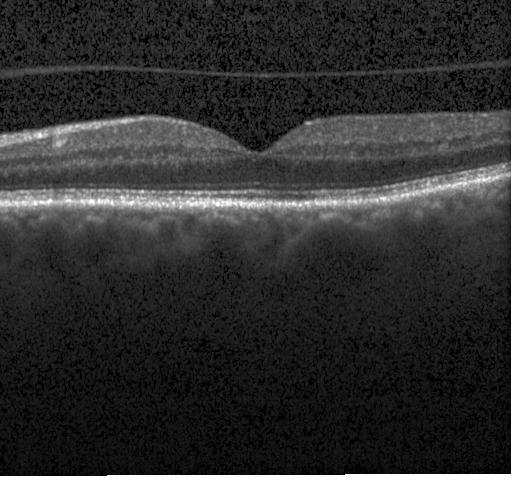 Macular OCT: no CNV, no DME, and no drusen.